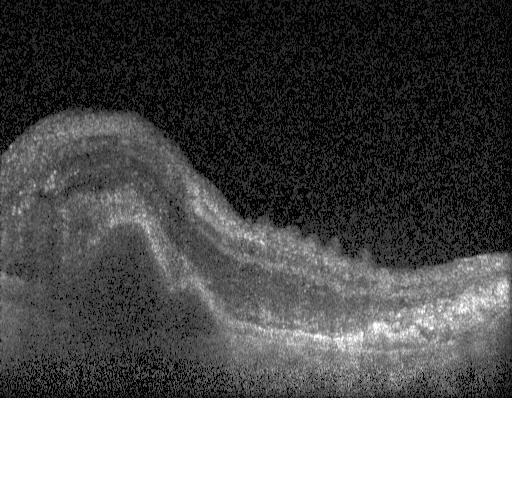 OCT B-scan showing choroidal neovascularization.